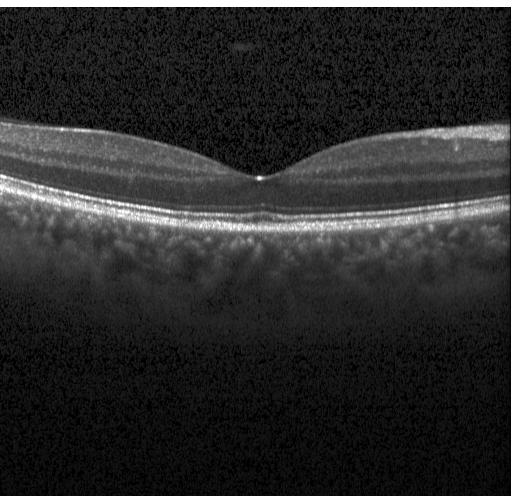 Macular OCT demonstrating no evidence of choroidal neovascularization, diabetic macular edema, or drusen.